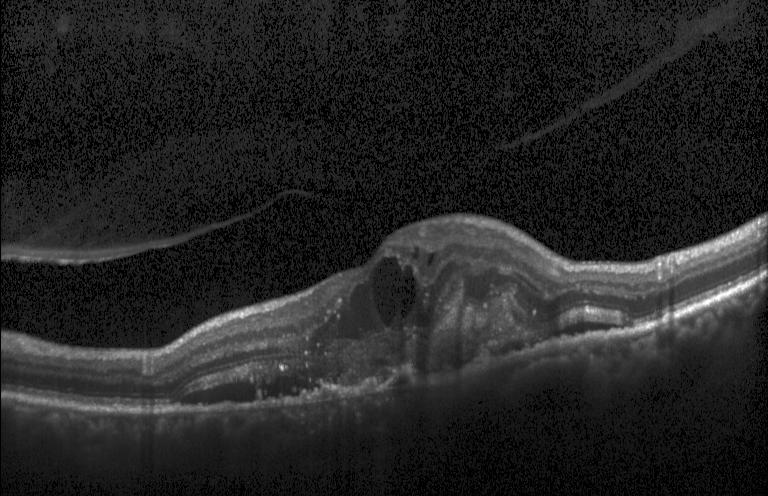

Finding: CNV.